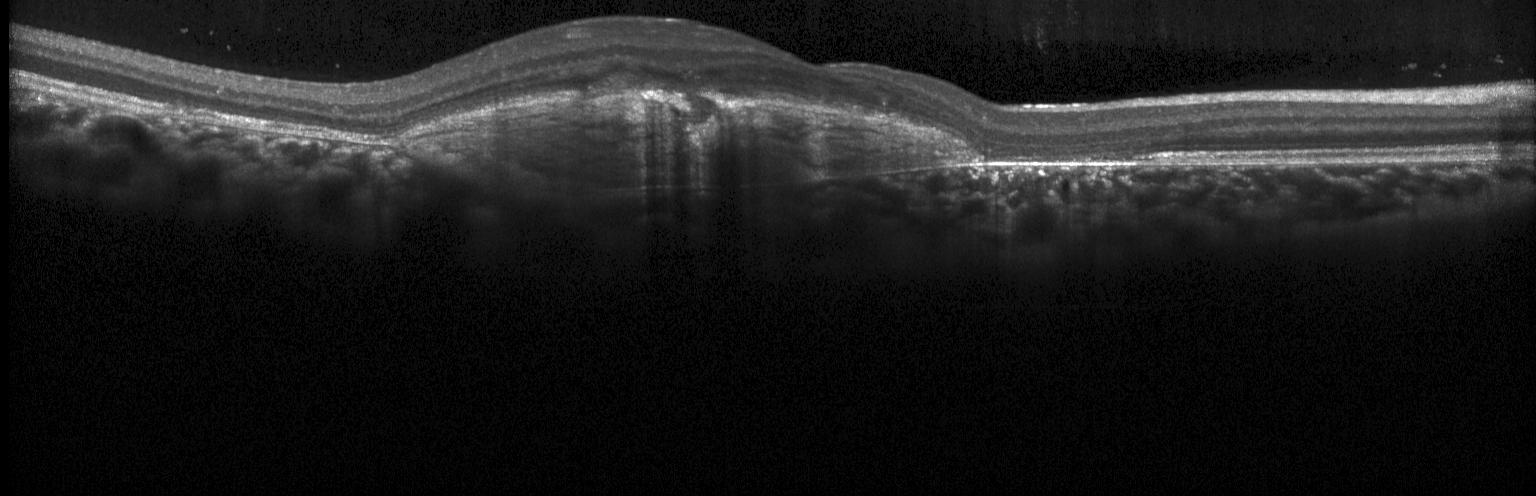

OCT B-scan; macular scan; Heidelberg Spectralis — Impression: a choroidal neovascular membrane.